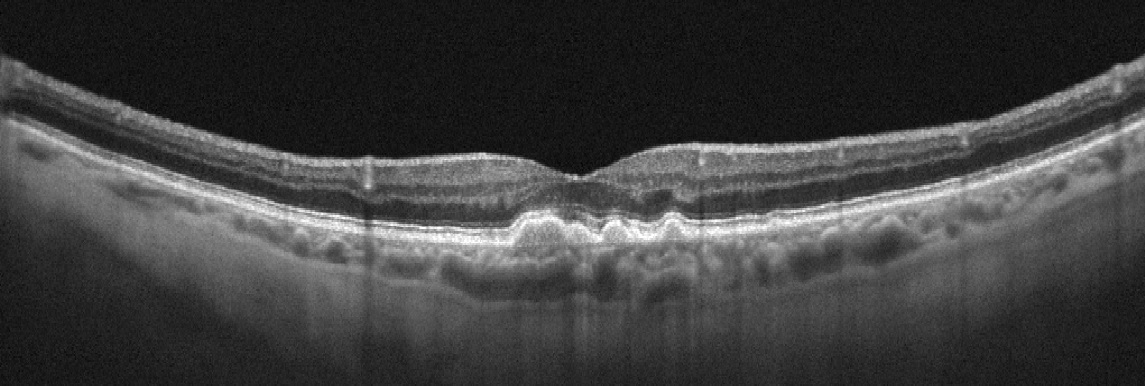 Macular scan. Retinal OCT B-scan. Acquired on an Optovue Avanti RTVue XR. This B-scan demonstrates AMD.